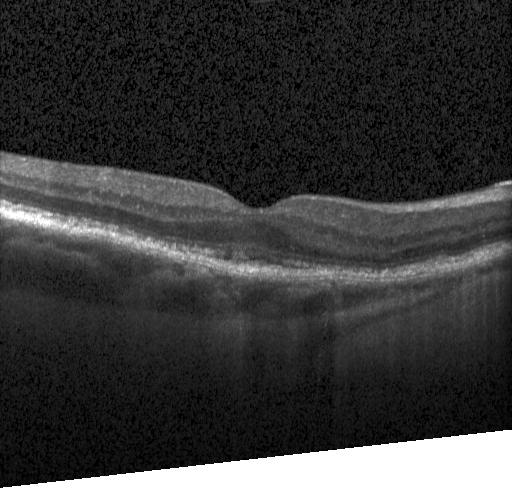 OCT B-scan. Finding: choroidal neovascularization.